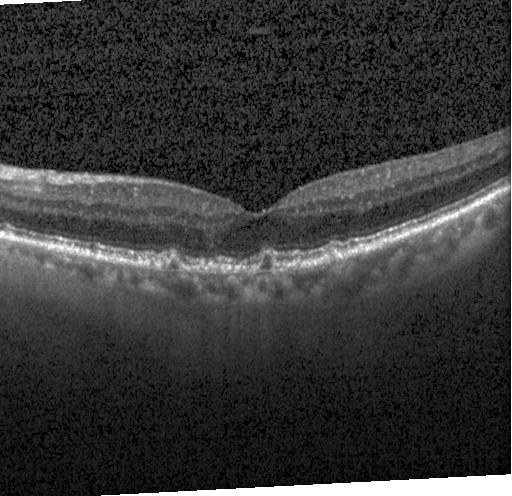

Optical coherence tomography scan, horizontal scan through the fovea, acquired on a Heidelberg Spectralis. Diagnosis: a choroidal neovascular membrane.